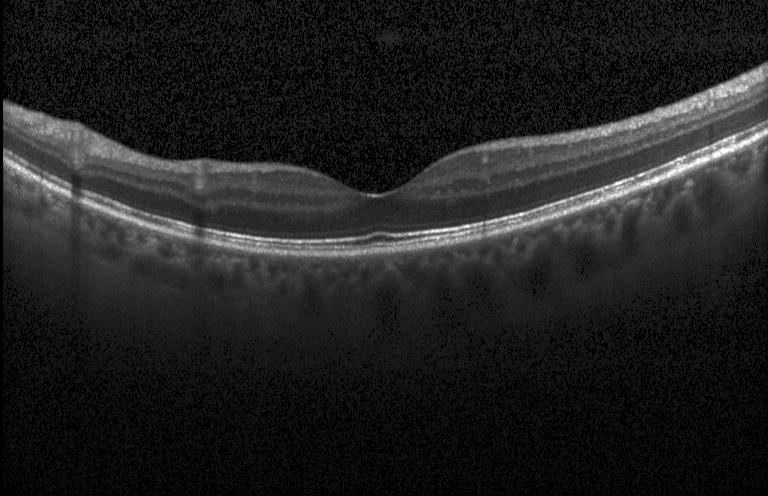
Retinal OCT B-scan · Heidelberg Spectralis · fovea-centered — OCT finding: no choroidal neovascularization, no diabetic macular edema, and no drusen.